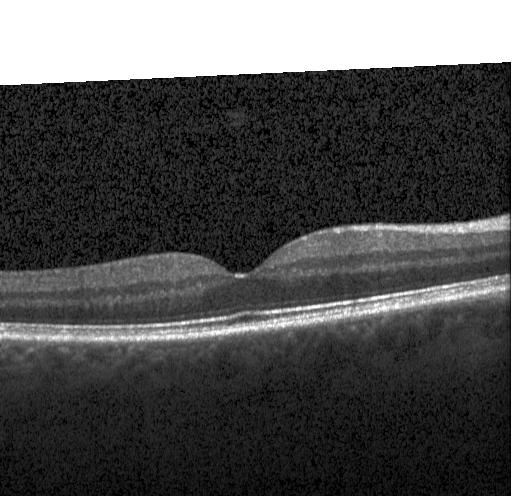 Dx: neither choroidal neovascularization, diabetic macular edema, nor drusen.